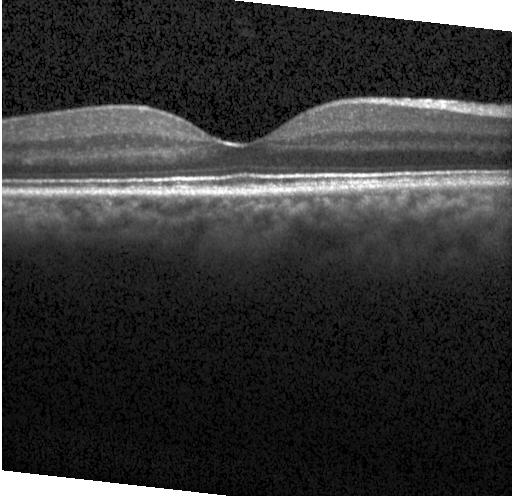
Spectral-domain OCT; retinal OCT cross-section; acquired on a Heidelberg Spectralis. OCT finding: no CNV, DME, or drusen.